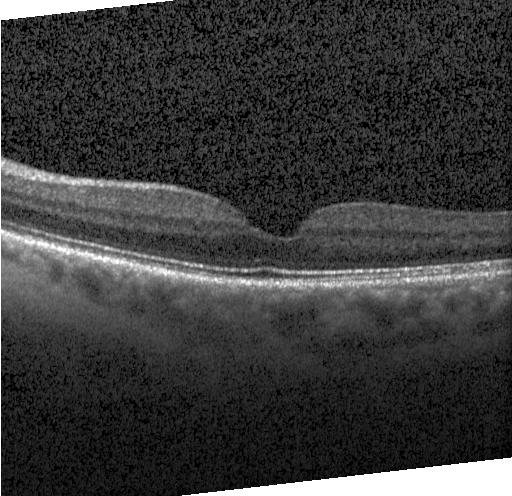

The scan shows no choroidal neovascularization, no diabetic macular edema, and no drusen.